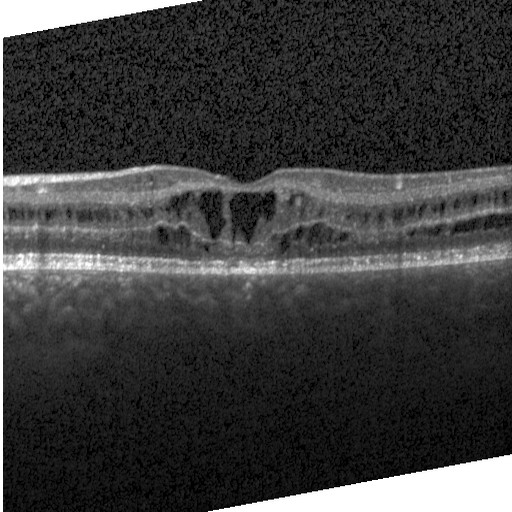
Optical coherence tomography scan, horizontal scan through the fovea — Diagnosis: diabetic macular edema.